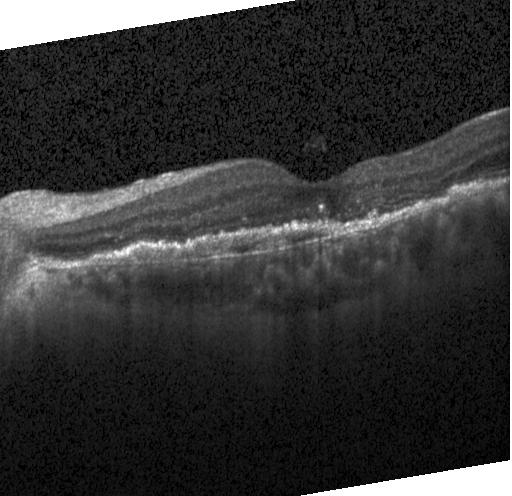

Optical coherence tomography B-scan, through the macula — Assessment: CNV.